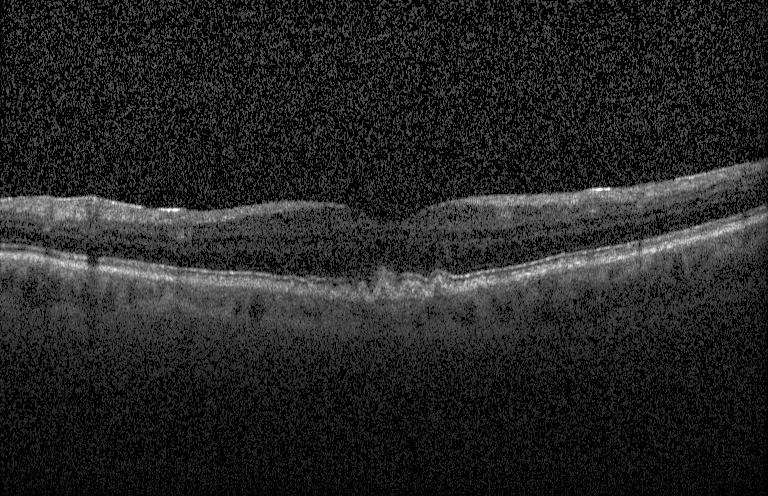

Finding: multiple drusen.